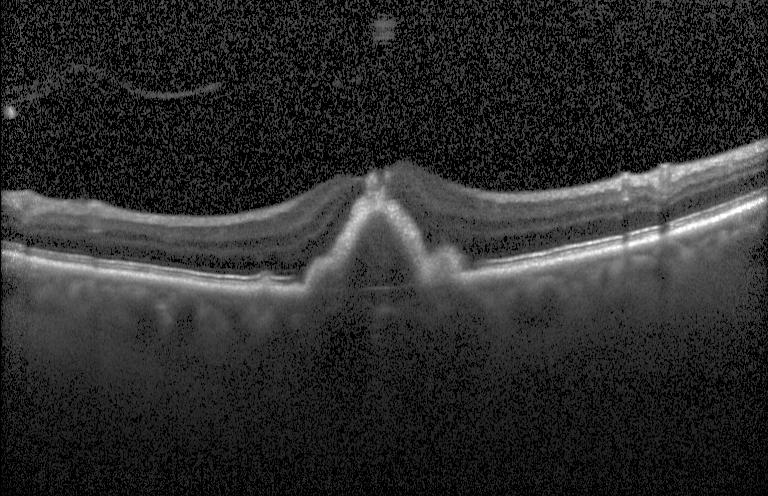
Macular OCT: a choroidal neovascular membrane.